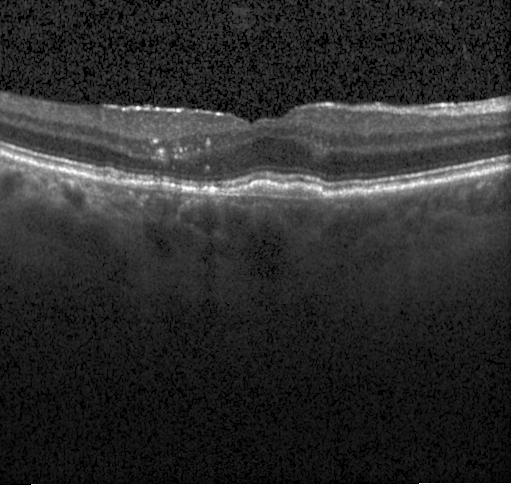
Optical coherence tomography B-scan.
Diagnosis: a choroidal neovascular membrane.